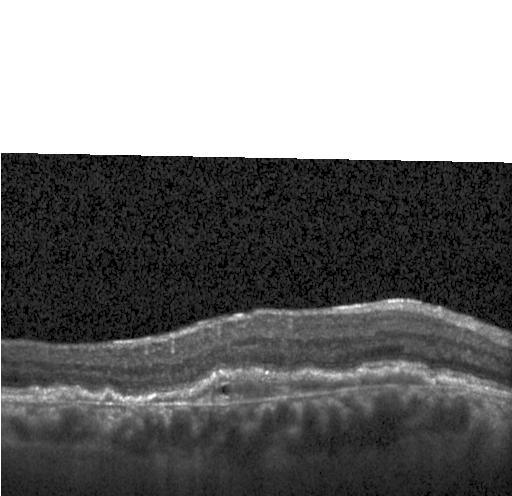
Finding: choroidal neovascularization (CNV).